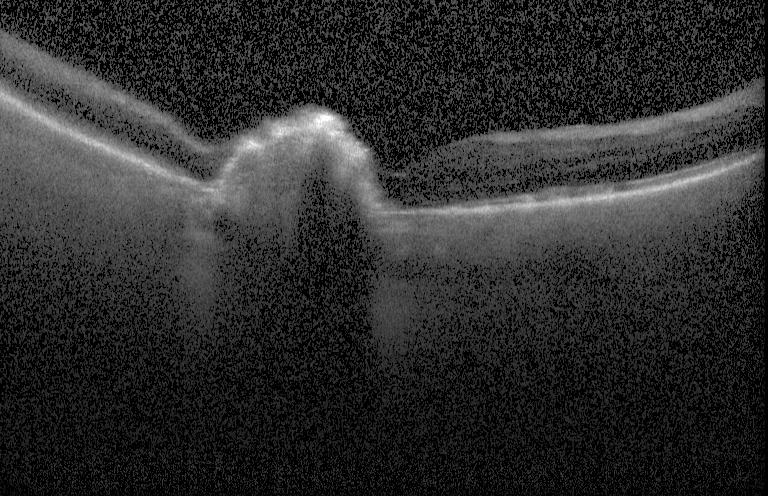

Retinal OCT cross-section, Heidelberg Spectralis OCT system. Assessment: choroidal neovascularization (CNV).